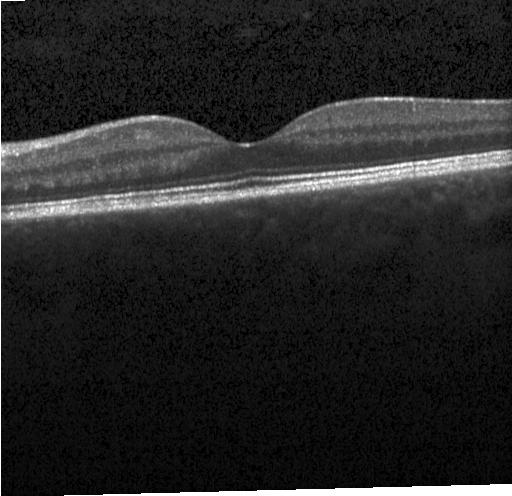
OCT B-scan · SD-OCT · horizontal scan through the fovea
No evidence of choroidal neovascularization, diabetic macular edema, or drusen.